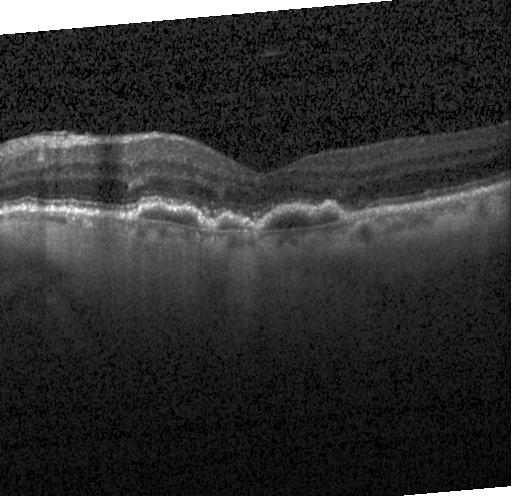

Horizontal scan through the fovea; spectral-domain OCT; optical coherence tomography scan; Heidelberg Spectralis — Dx: a choroidal neovascular membrane.